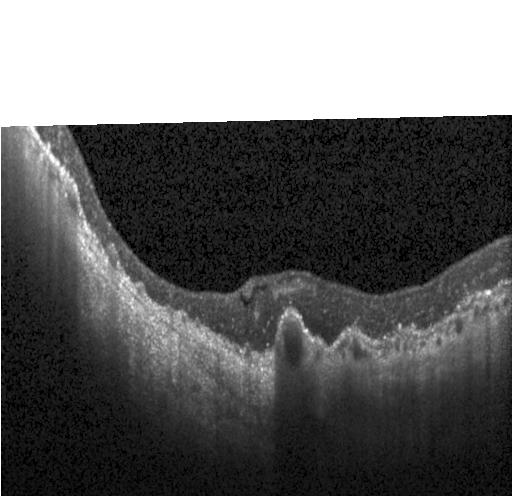 Retinal OCT cross-section. Horizontal scan through the fovea — OCT finding: choroidal neovascularization.